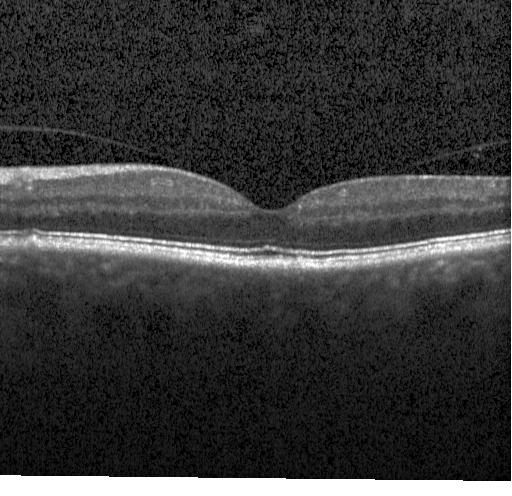
Spectral-domain optical coherence tomography. Macular scan. Instrument: Heidelberg Spectralis. Optical coherence tomography B-scan. Finding: no choroidal neovascularization, no diabetic macular edema, and no drusen.